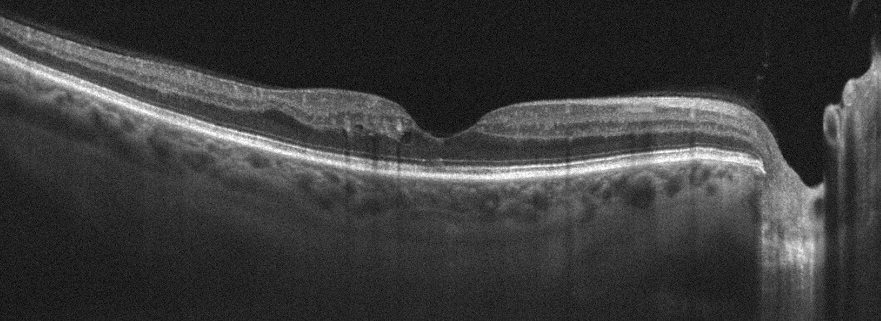

OCT scan showing DME.